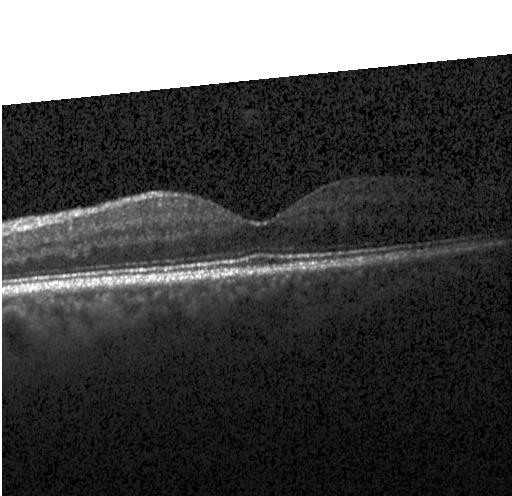

Assessment: no choroidal neovascularization, diabetic macular edema, or drusen.